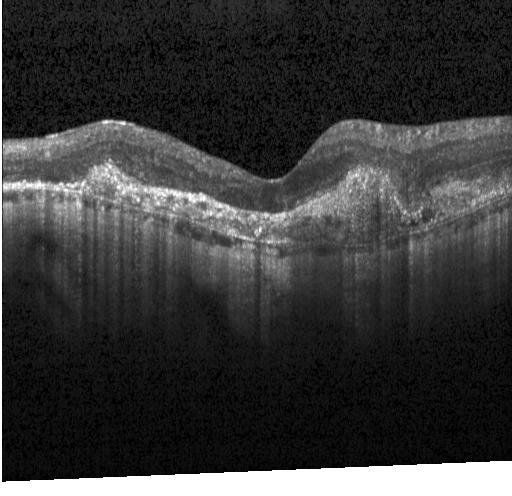
Retinal OCT B-scan · instrument: Heidelberg Spectralis.
Finding: choroidal neovascularization (CNV).